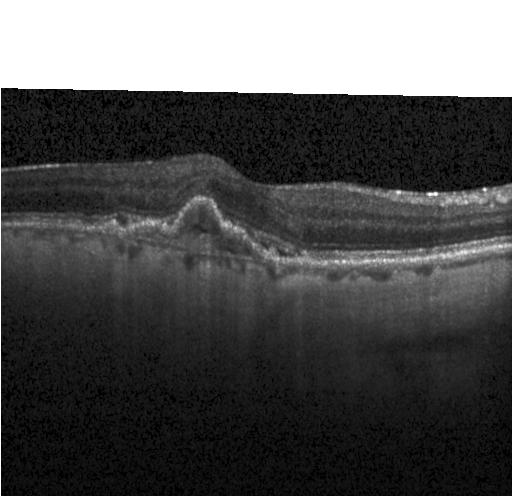
SD-OCT. Retinal OCT cross-section. A choroidal neovascular membrane.